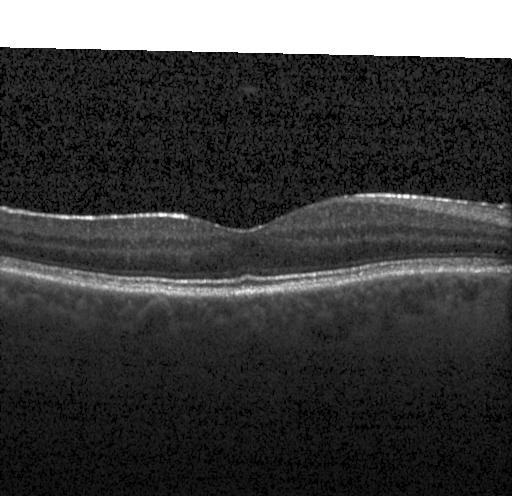
Spectral-domain OCT. Optical coherence tomography B-scan. Through the macula. Diagnosis: no choroidal neovascularization, no diabetic macular edema, and no drusen.